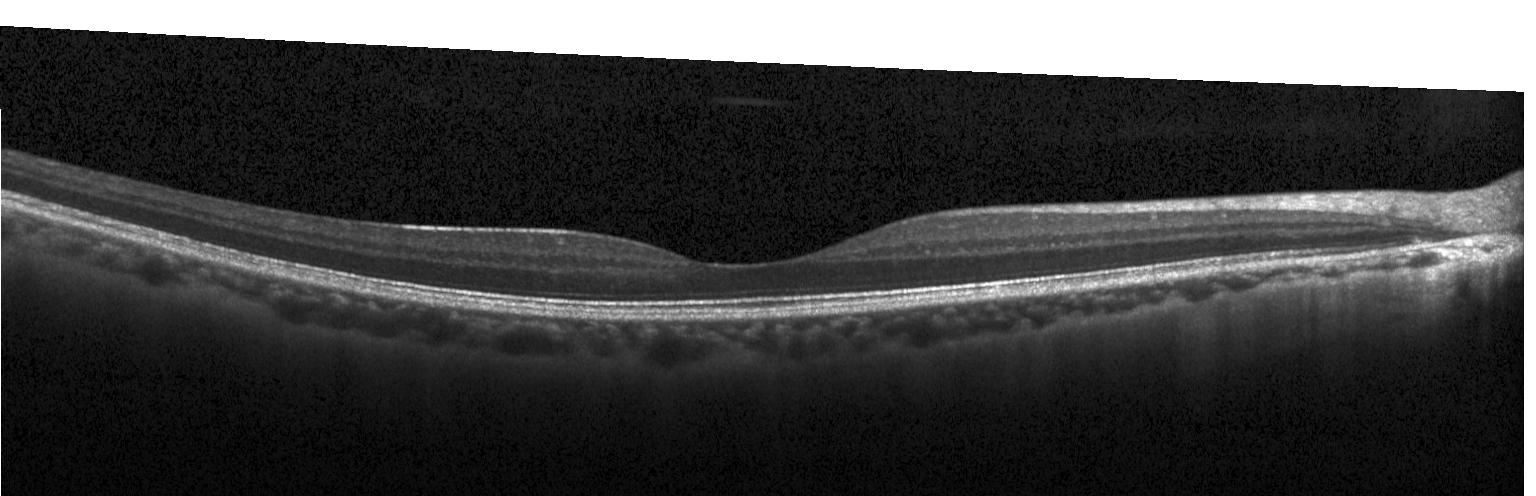 Acquired on a Heidelberg Spectralis. Spectral-domain optical coherence tomography. Centered on the fovea. Optical coherence tomography B-scan.
This B-scan demonstrates no choroidal neovascularization, diabetic macular edema, or drusen.